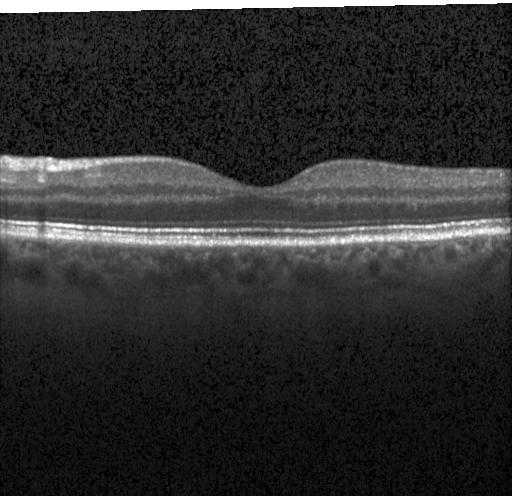

Retinal OCT cross-section — Macular OCT: no CNV, no DME, and no drusen.